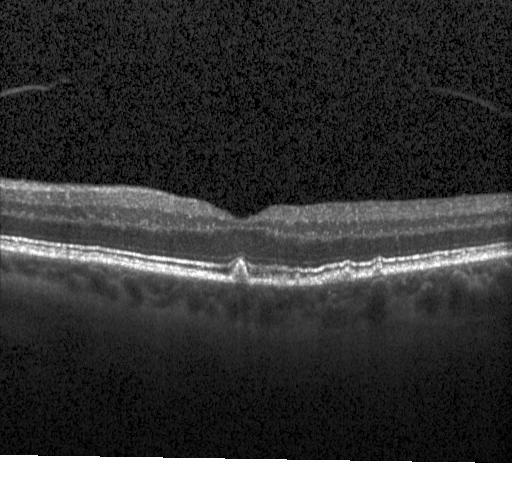
Acquired on a Heidelberg Spectralis, SD-OCT, retinal OCT cross-section.
Sub-RPE drusenoid deposits.